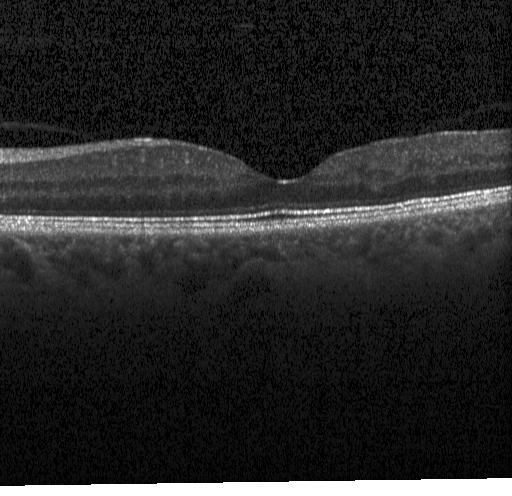
Diagnosis: neither choroidal neovascularization, diabetic macular edema, nor drusen.